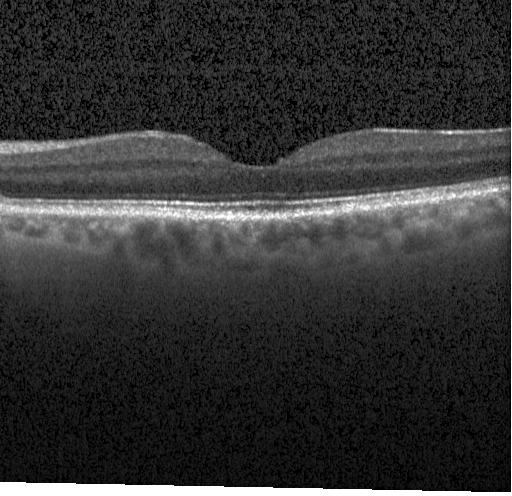 Optical coherence tomography scan.
This B-scan demonstrates no choroidal neovascularization, diabetic macular edema, or drusen.